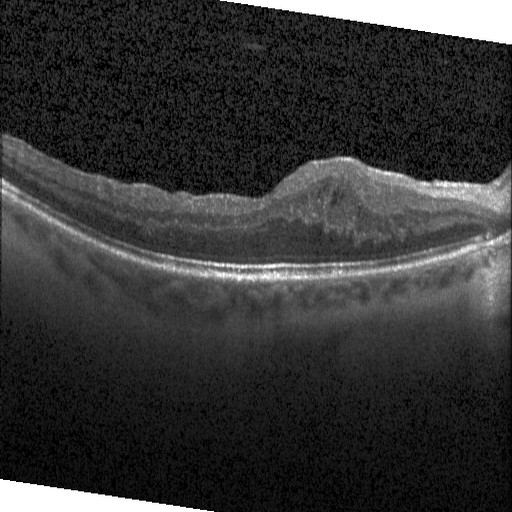

Finding: diabetic macular edema (DME).